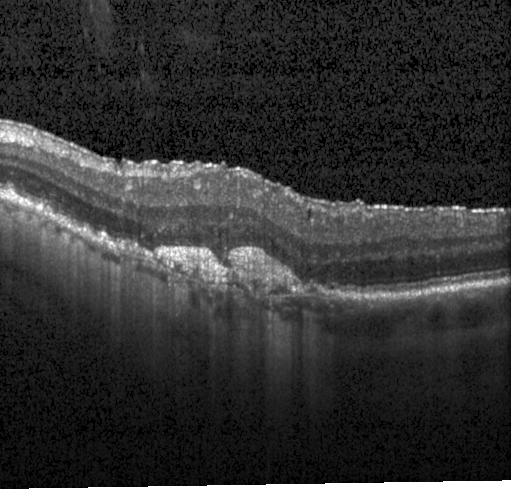
Macular OCT: CNV.